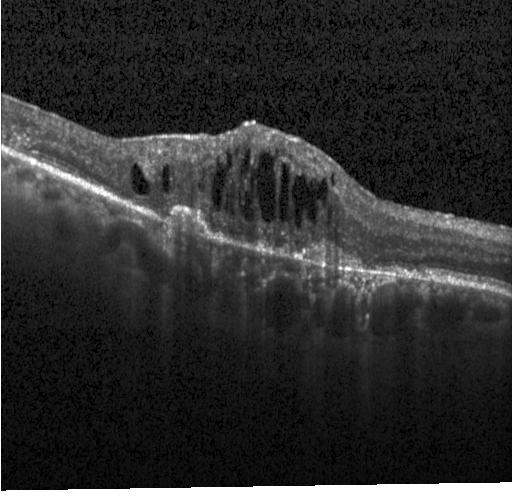

This B-scan demonstrates CNV.